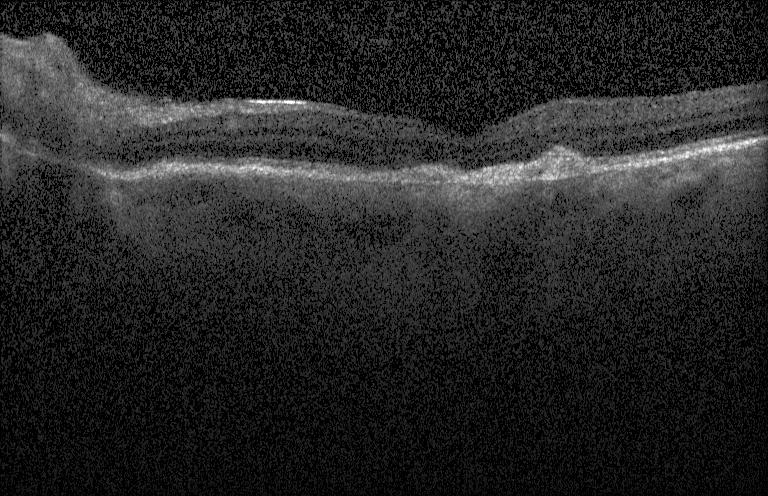 Macular scan, retinal OCT B-scan
Assessment: a choroidal neovascular membrane.